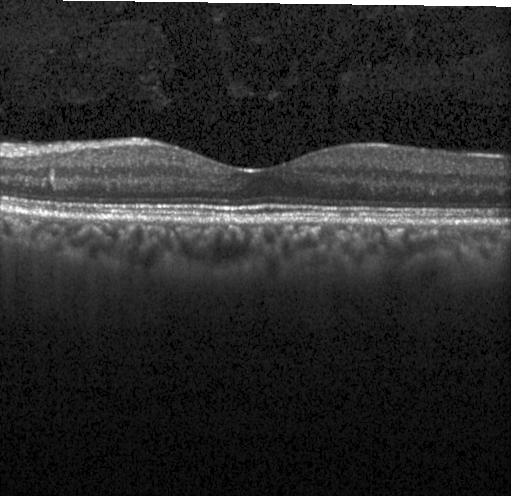
SD-OCT; optical coherence tomography B-scan; acquired on a Heidelberg Spectralis; through the macula
Finding: no evidence of CNV, DME, or drusen.